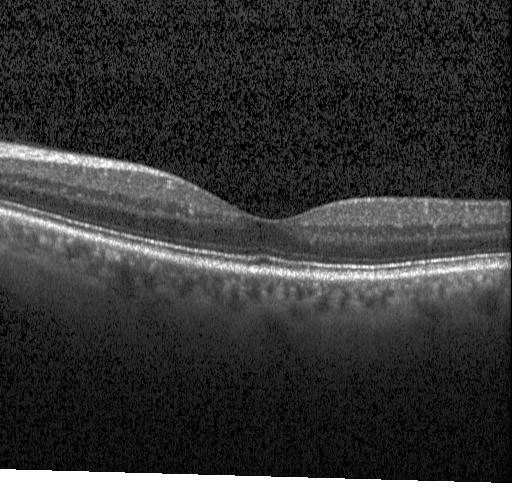 Through the macula · spectral-domain optical coherence tomography · OCT B-scan · Heidelberg Spectralis. OCT finding: no evidence of choroidal neovascularization, diabetic macular edema, or drusen.